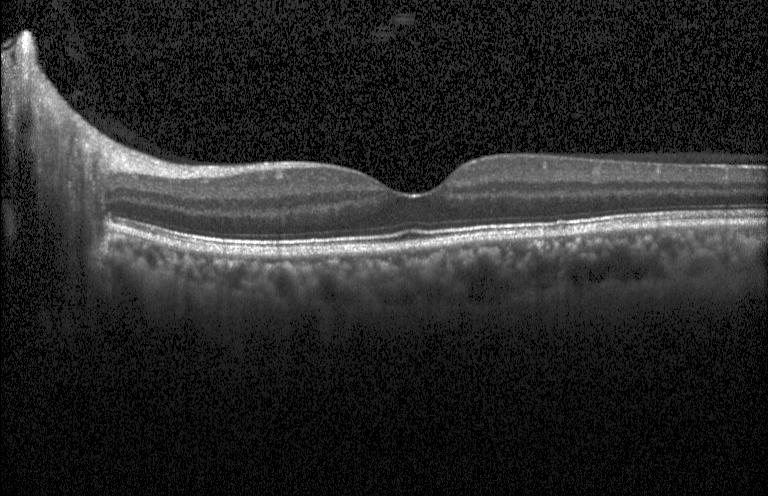
Macular scan. SD-OCT. OCT B-scan. Heidelberg Spectralis OCT system. Finding: neither choroidal neovascularization, diabetic macular edema, nor drusen.